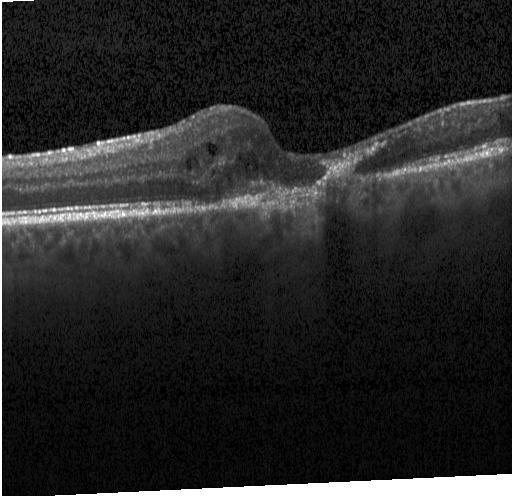

Diagnosis: choroidal neovascularization.